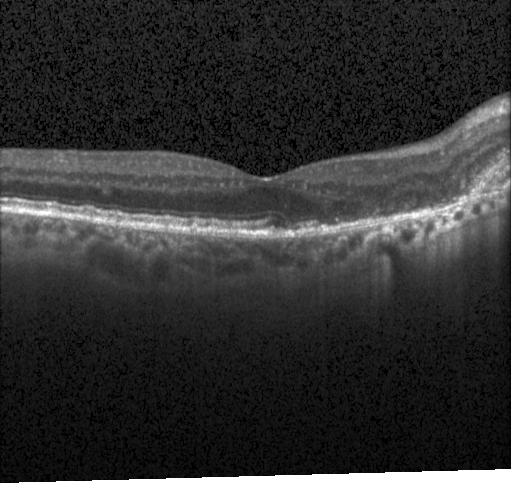

Retinal OCT cross-section
A choroidal neovascular membrane.